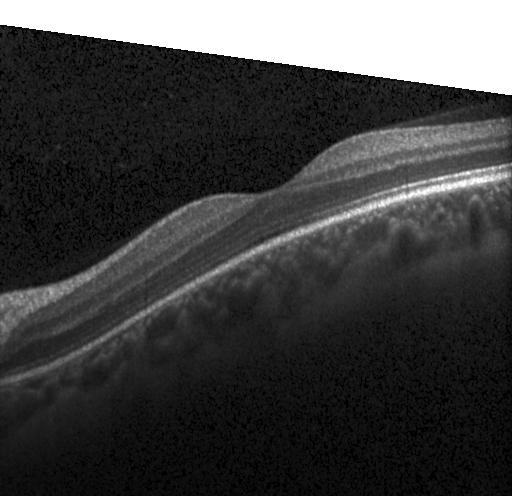
Spectral-domain optical coherence tomography; instrument: Heidelberg Spectralis; retinal OCT cross-section; macular scan — Assessment: no CNV, DME, or drusen.